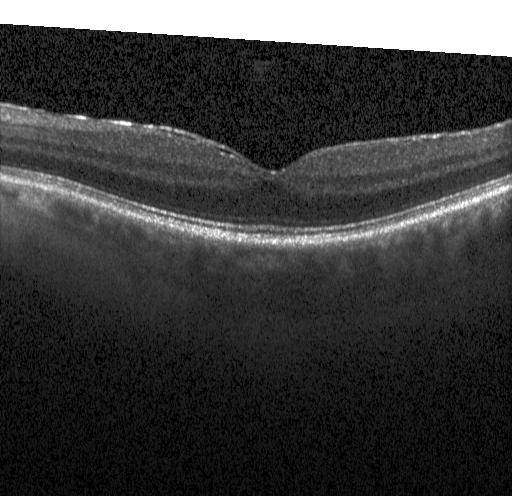 Dx: no evidence of choroidal neovascularization, diabetic macular edema, or drusen.